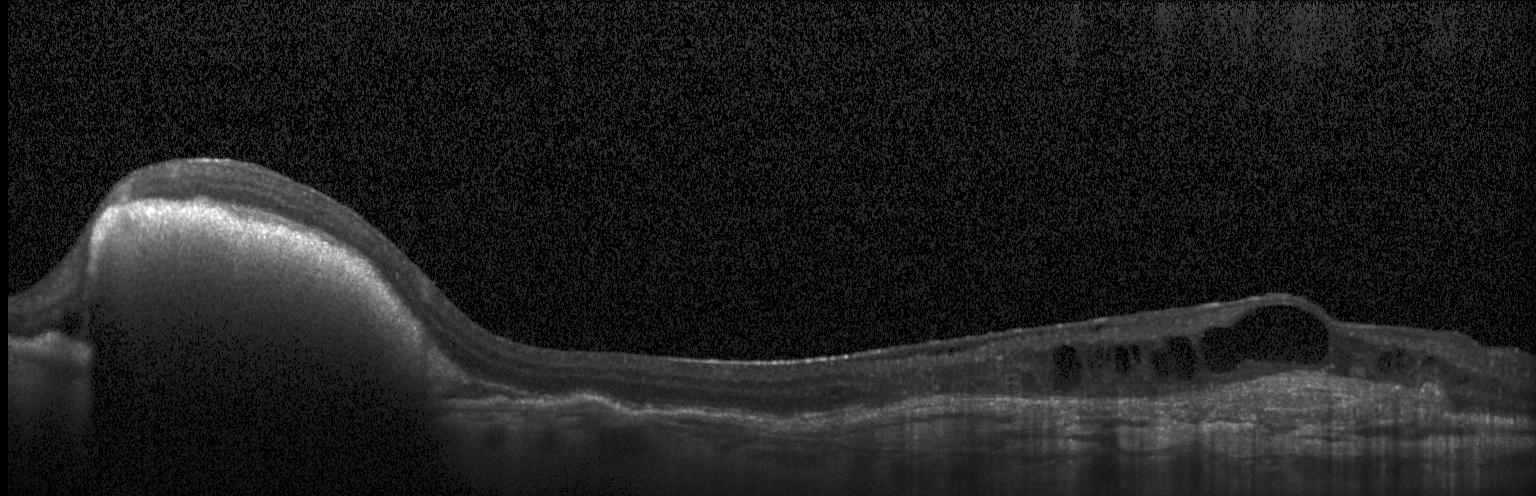

OCT scan showing choroidal neovascularization (CNV).